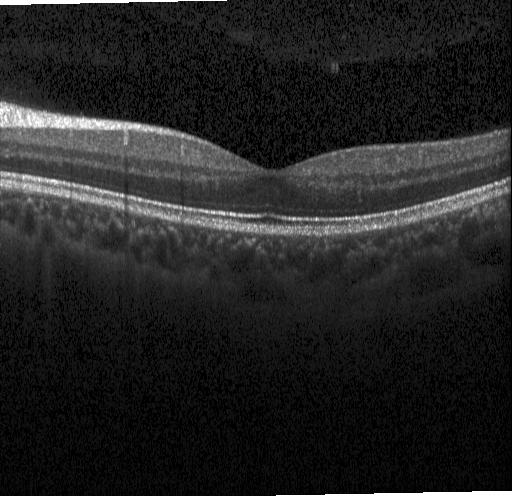 Finding: no choroidal neovascularization, no diabetic macular edema, and no drusen.